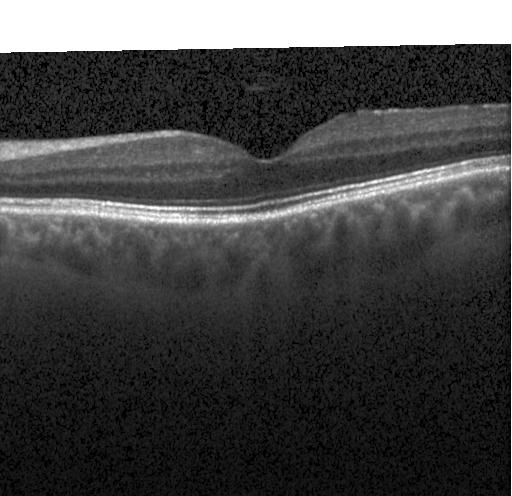

Spectral-domain optical coherence tomography. Optical coherence tomography B-scan — Impression: no choroidal neovascularization, no diabetic macular edema, and no drusen.